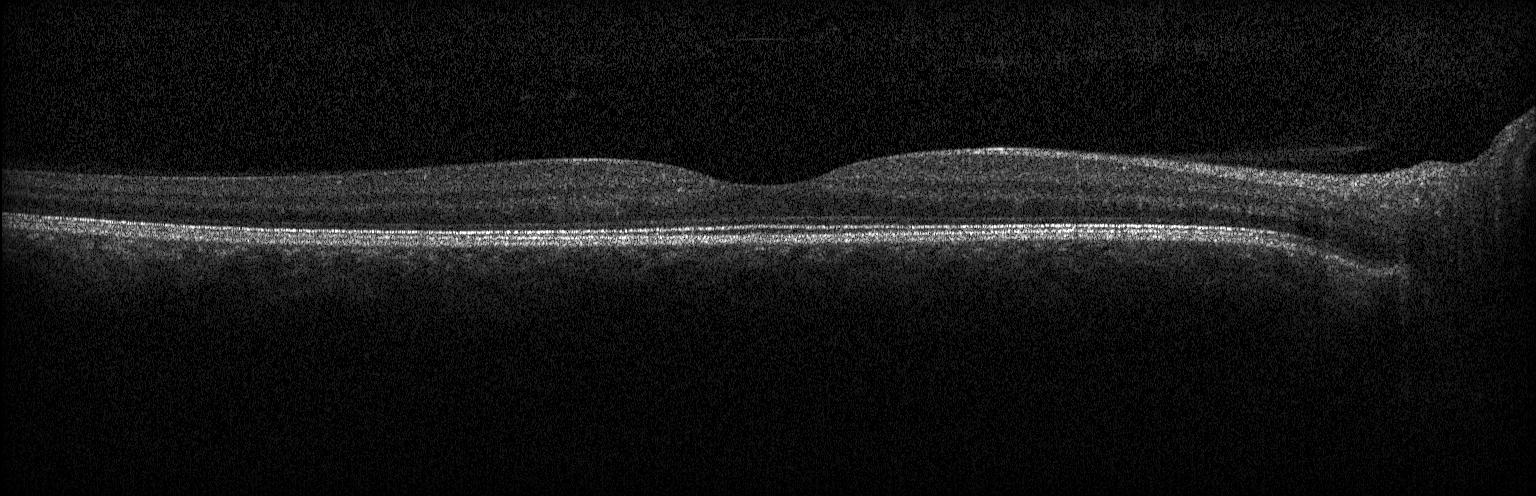 Centered on the fovea. Optical coherence tomography B-scan. SD-OCT.
Finding: no evidence of choroidal neovascularization, diabetic macular edema, or drusen.